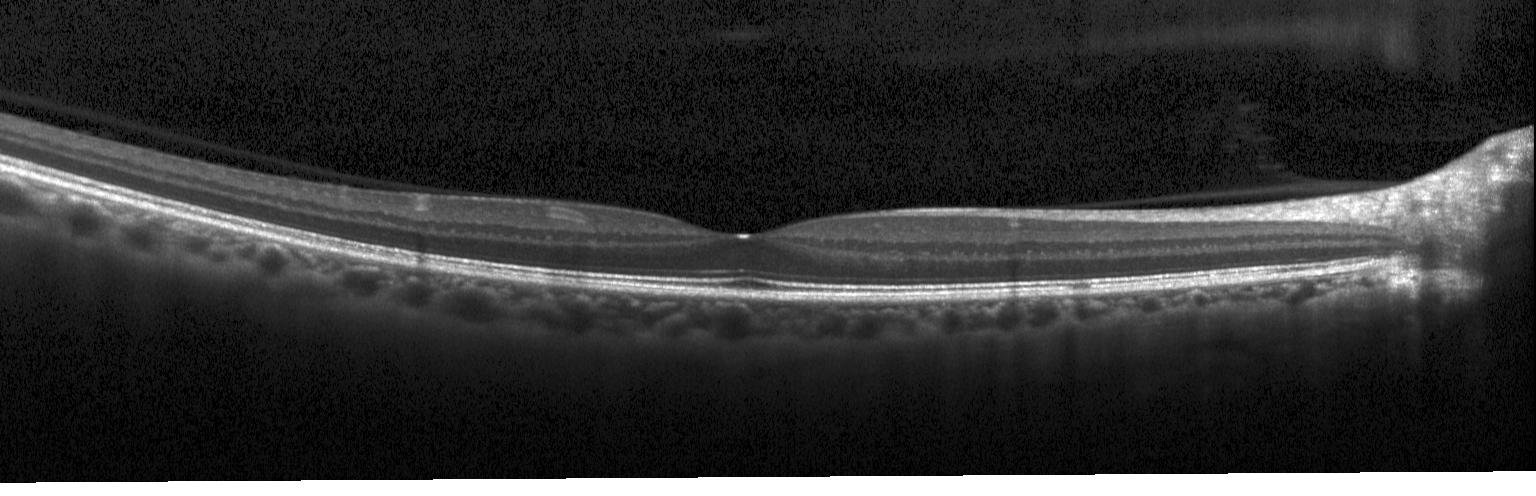
Dx: no CNV, DME, or drusen.